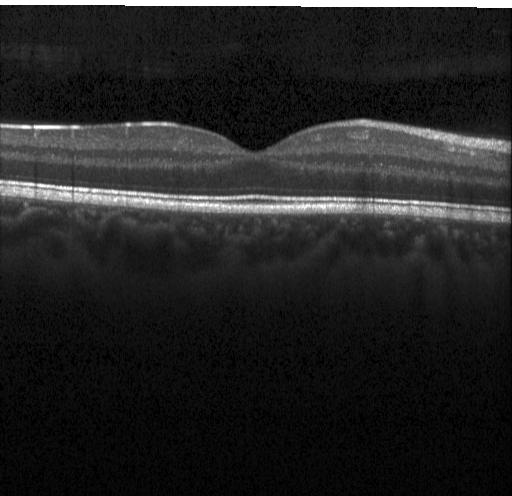

Impression: no choroidal neovascularization, no diabetic macular edema, and no drusen.